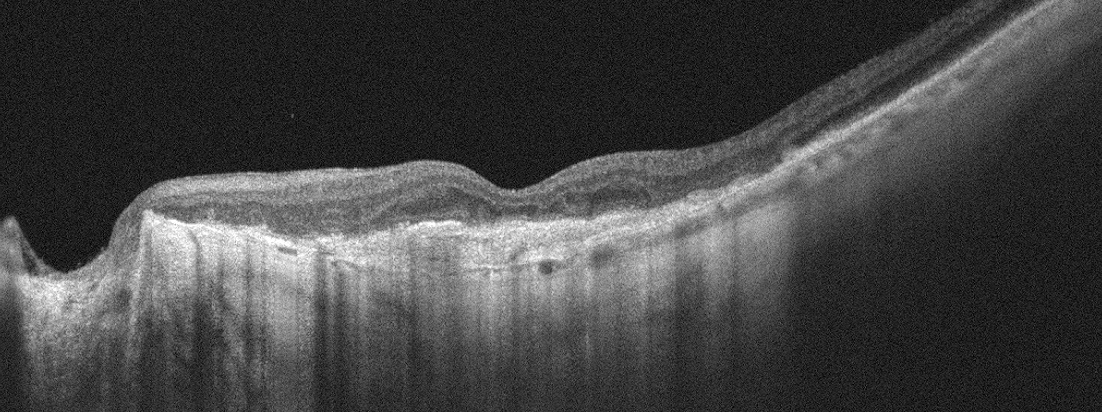 Instrument: Optovue Avanti RTVue XR; macular scan; optical coherence tomography B-scan. Diagnosis: AMD.